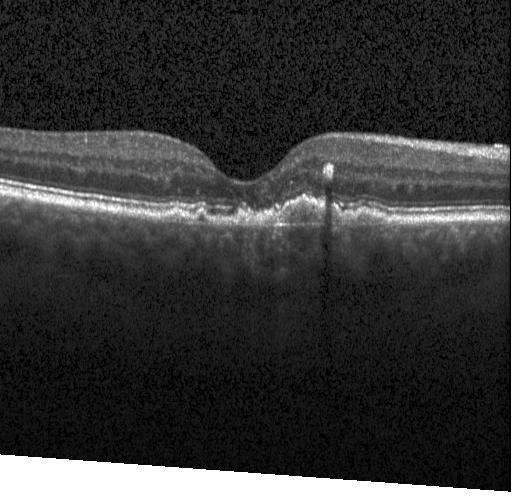 Assessment: choroidal neovascularization.